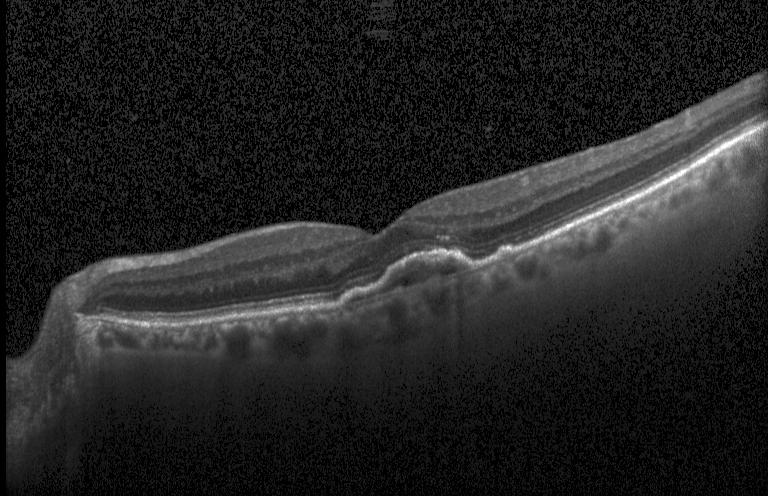

Dx: choroidal neovascularization.